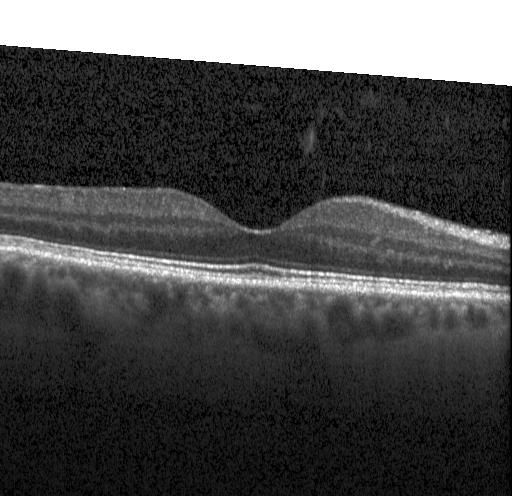

Finding: neither CNV, DME, nor drusen.